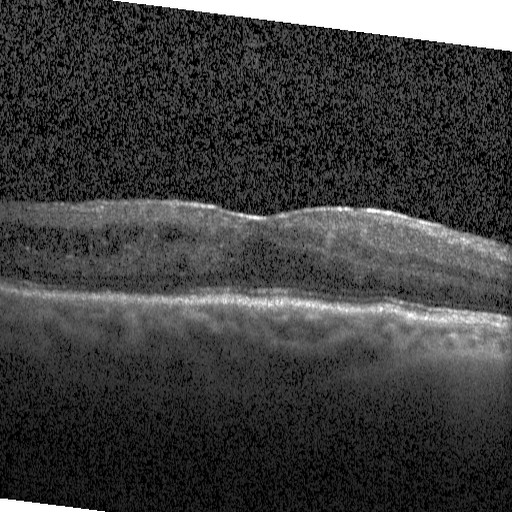 Optical coherence tomography scan — Macular OCT: DME.